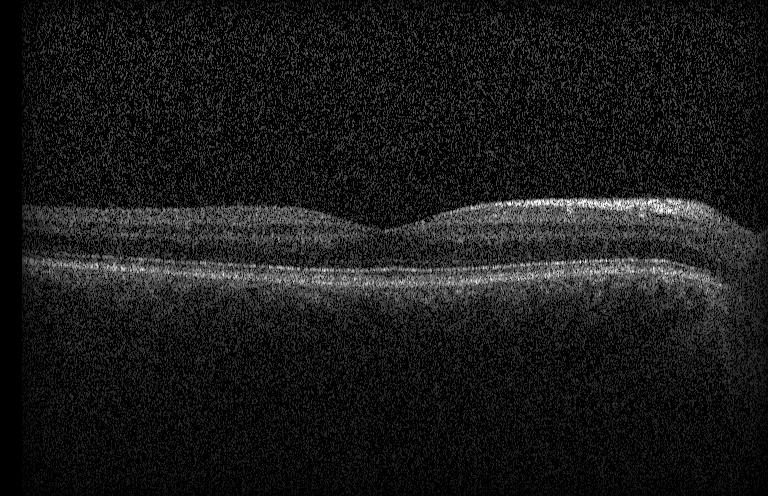
Spectral-domain OCT · centered on the fovea · OCT line scan · Heidelberg Spectralis OCT system.
This B-scan demonstrates neither choroidal neovascularization, diabetic macular edema, nor drusen.